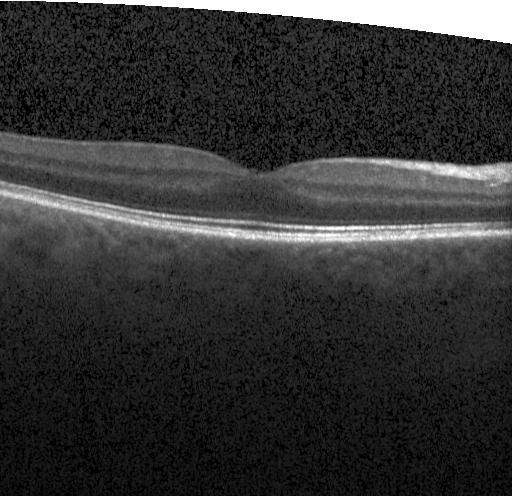 Retinal OCT B-scan, horizontal scan through the fovea — Diagnosis: no evidence of choroidal neovascularization, diabetic macular edema, or drusen.